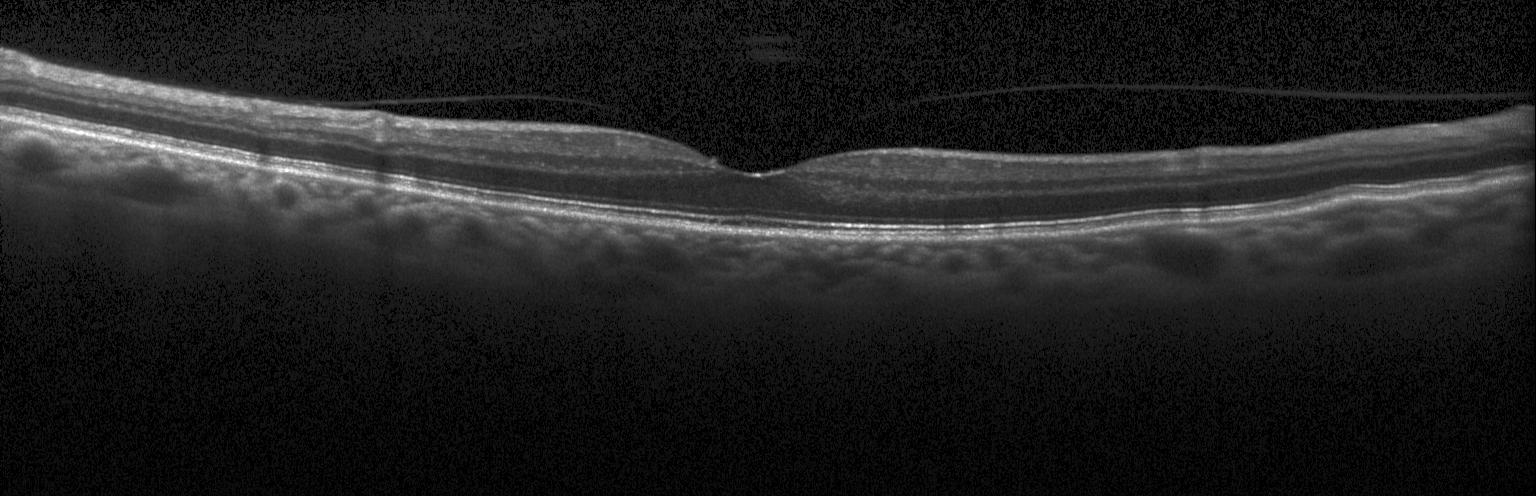 The scan shows no evidence of choroidal neovascularization, diabetic macular edema, or drusen.